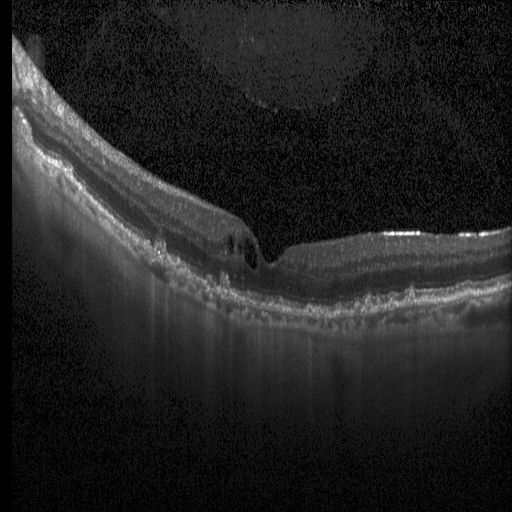

Diagnosis: diabetic macular edema (DME).